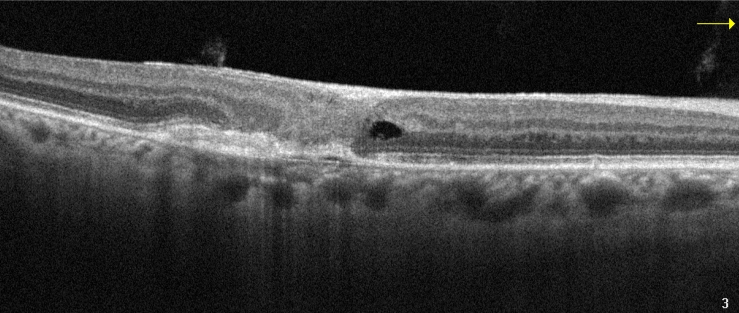 Retinal OCT B-scan; acquired on an Optovue Avanti RTVue XR
Assessment: age-related macular degeneration (AMD).